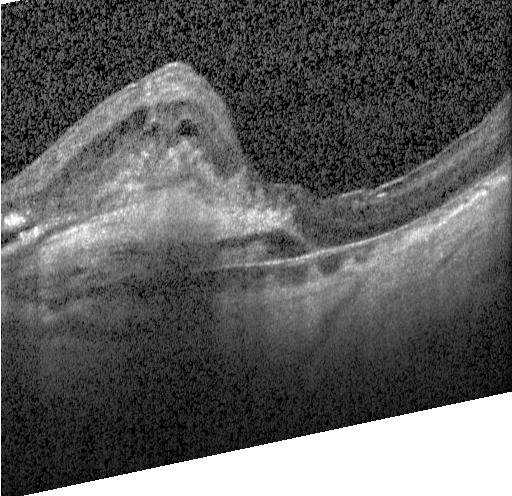
Optical coherence tomography scan, horizontal scan through the fovea, Heidelberg Spectralis OCT system, spectral-domain optical coherence tomography.
A choroidal neovascular membrane.